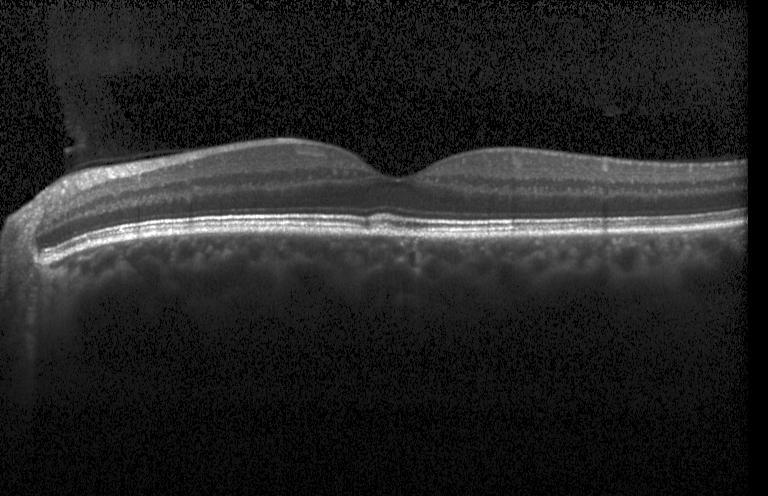 OCT finding: no choroidal neovascularization, diabetic macular edema, or drusen.